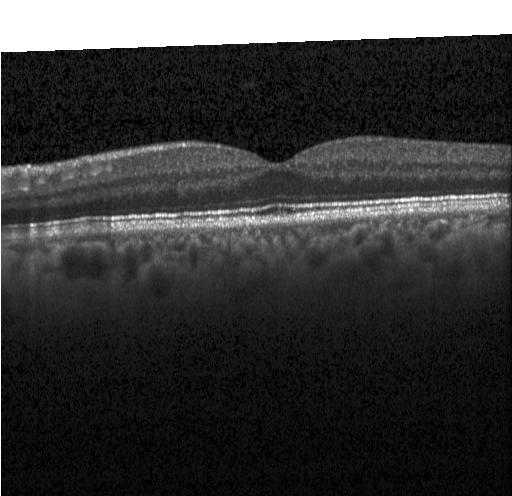 Centered on the fovea · retinal OCT B-scan · acquired on a Heidelberg Spectralis. Assessment: no choroidal neovascularization, diabetic macular edema, or drusen.